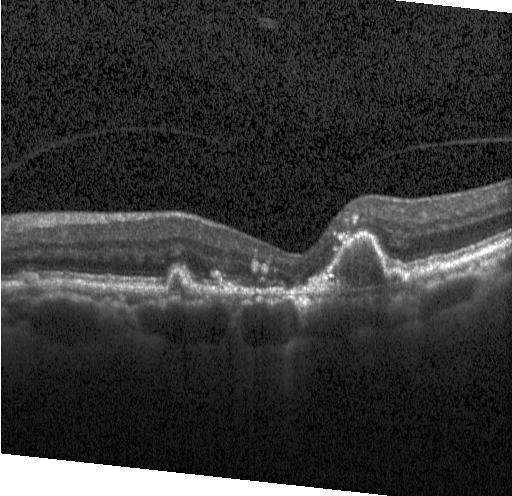 Diagnosis: a choroidal neovascular membrane.